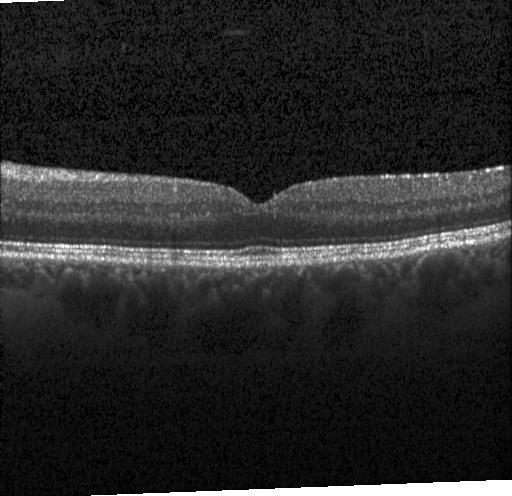 Retinal OCT cross-section.
No evidence of CNV, DME, or drusen.